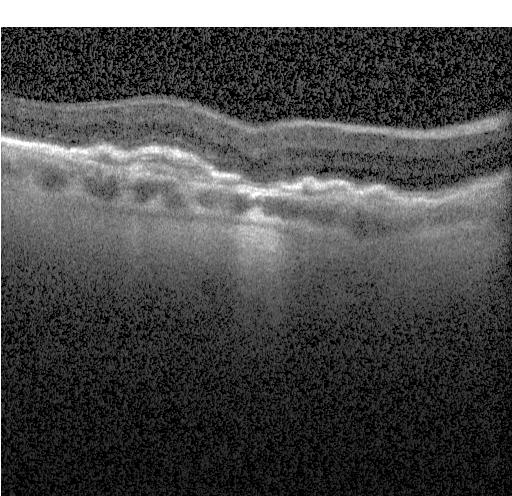

Spectral-domain OCT · instrument: Heidelberg Spectralis · retinal OCT B-scan · fovea-centered — Macular OCT: a choroidal neovascular membrane.